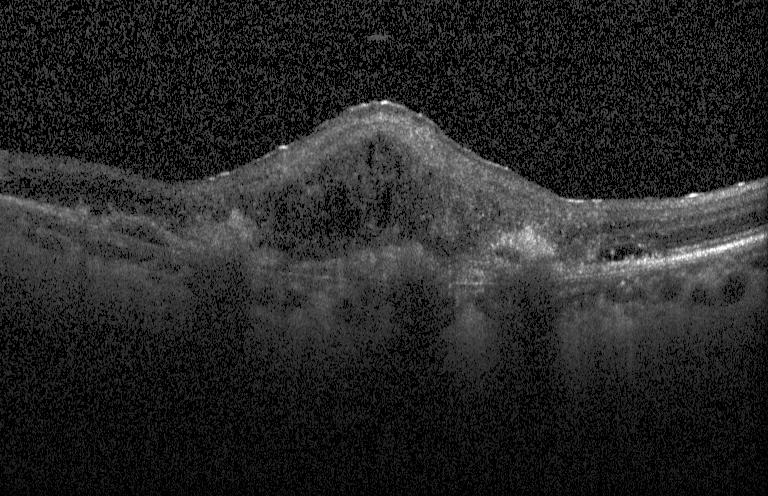
Spectral-domain optical coherence tomography. Optical coherence tomography B-scan. A choroidal neovascular membrane.